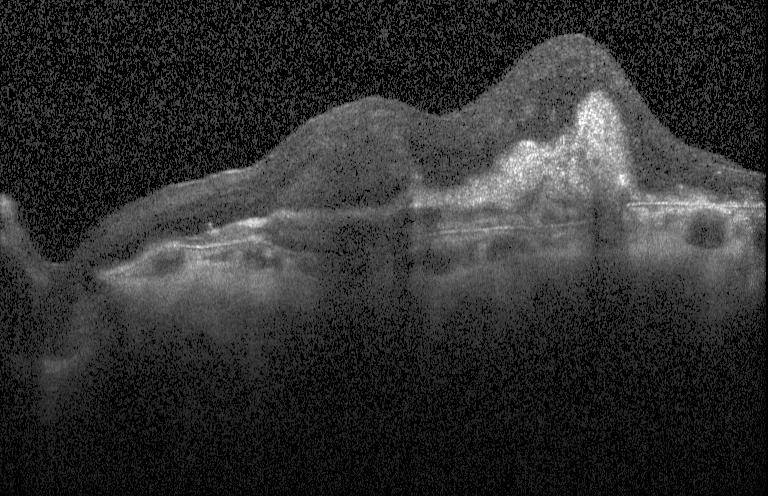

OCT B-scan · SD-OCT
OCT finding: a choroidal neovascular membrane.